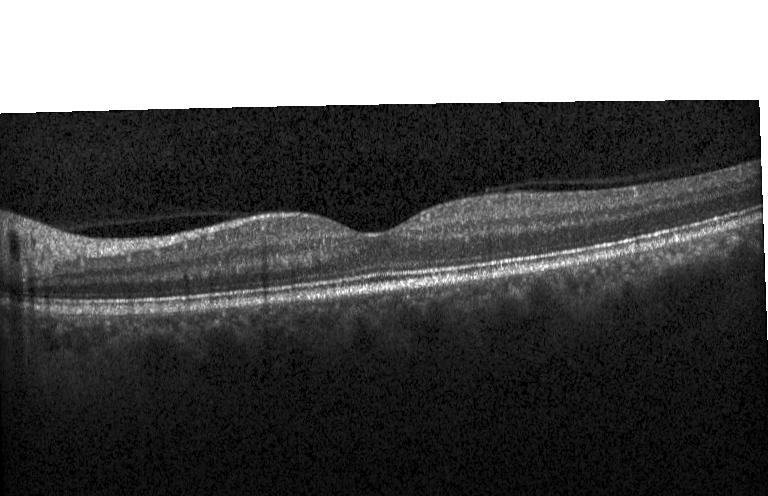

OCT line scan, SD-OCT, centered on the fovea — This B-scan demonstrates neither CNV, DME, nor drusen.